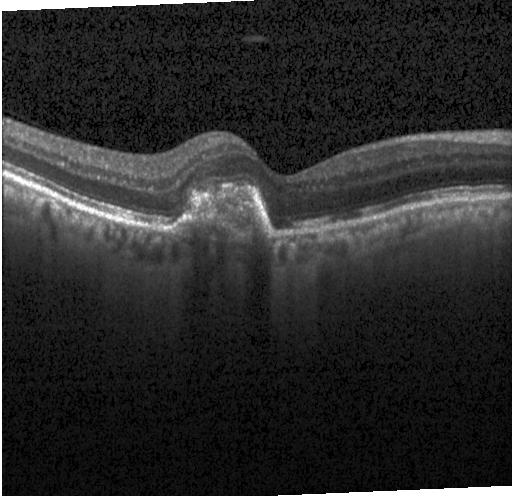 Optical coherence tomography B-scan, instrument: Heidelberg Spectralis, horizontal scan through the fovea. The scan shows a choroidal neovascular membrane.